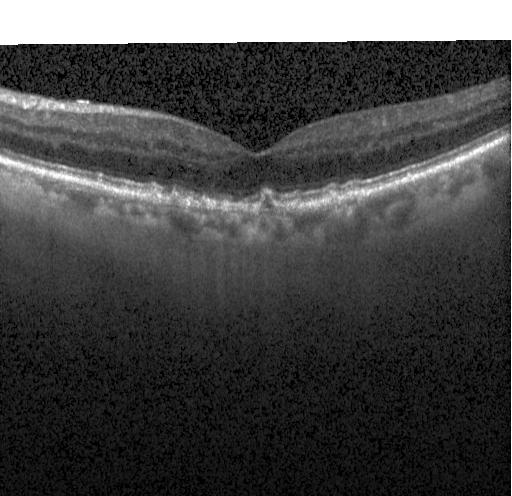 OCT B-scan; instrument: Heidelberg Spectralis; centered on the fovea
Assessment: multiple drusen.